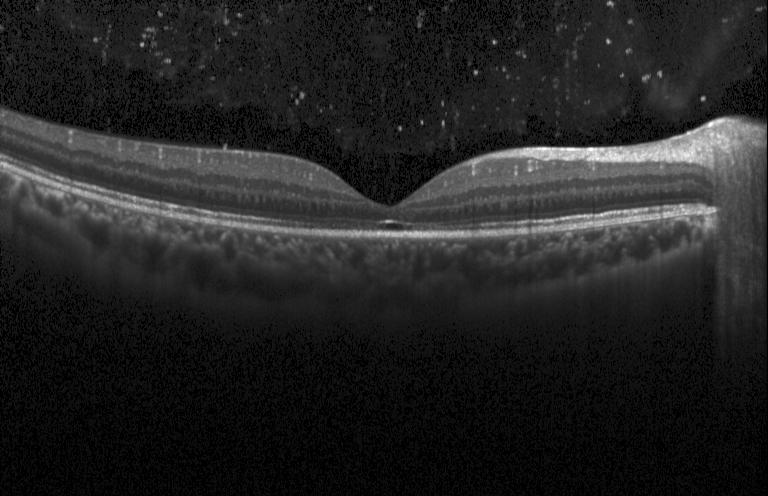
OCT finding: neither choroidal neovascularization, diabetic macular edema, nor drusen.